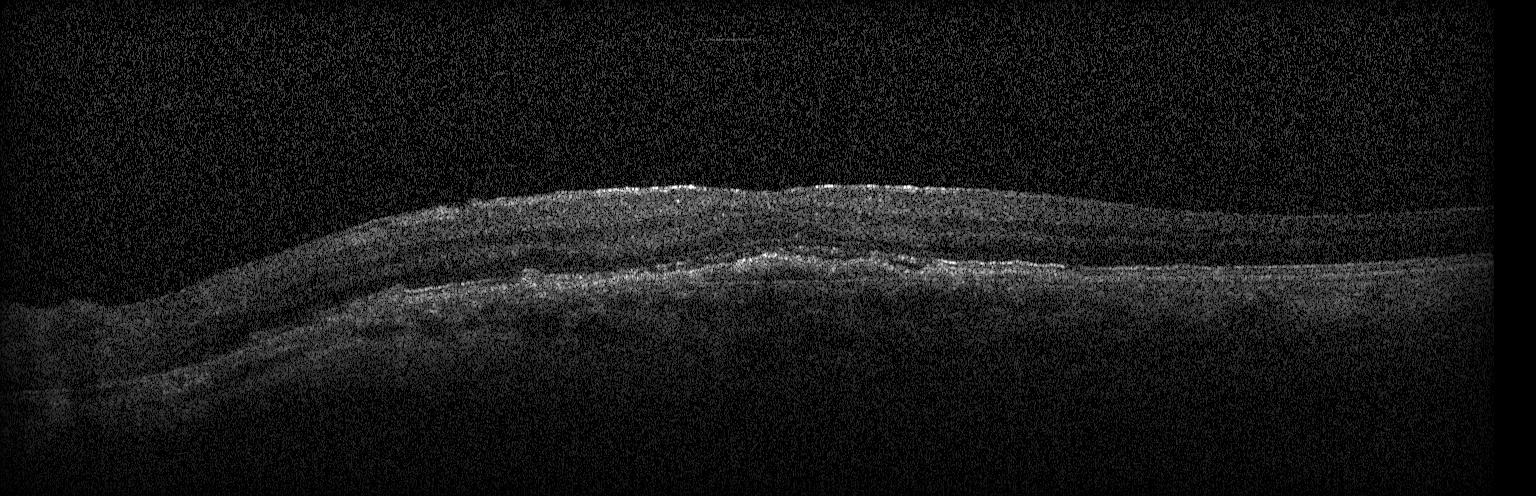 Instrument: Heidelberg Spectralis; spectral-domain optical coherence tomography; retinal OCT cross-section; fovea-centered. Assessment: choroidal neovascularization (CNV).